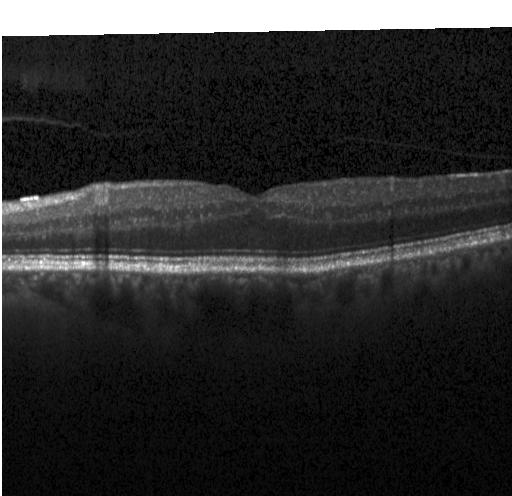
Neither CNV, DME, nor drusen.